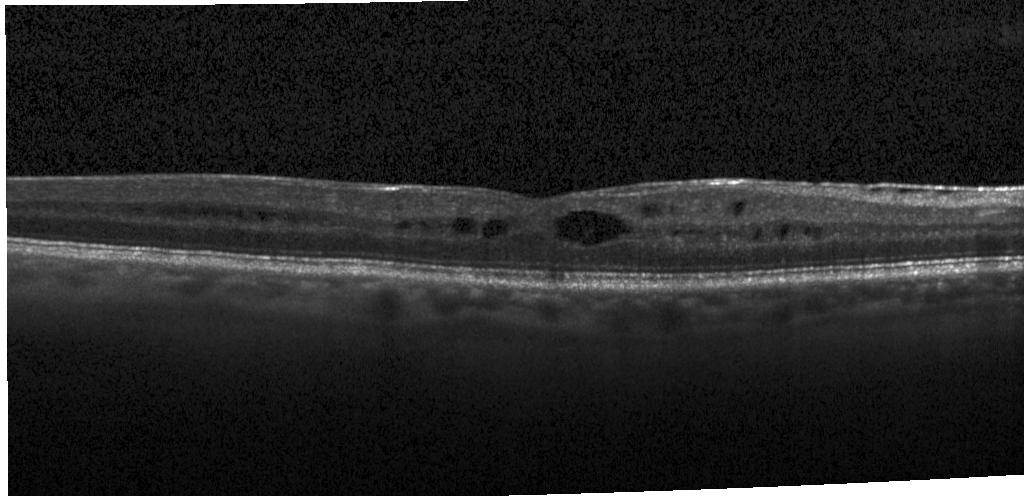
Impression: diabetic macular edema (DME).